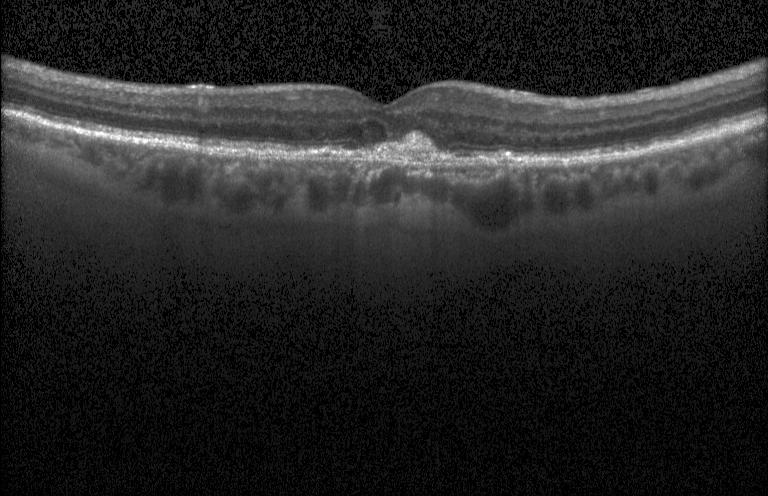 Heidelberg Spectralis OCT system. Spectral-domain optical coherence tomography. Macular scan. Retinal OCT B-scan.
Choroidal neovascularization (CNV).